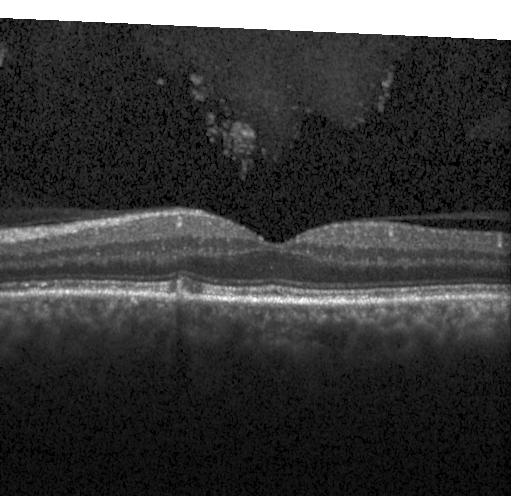 Dx: drusen.